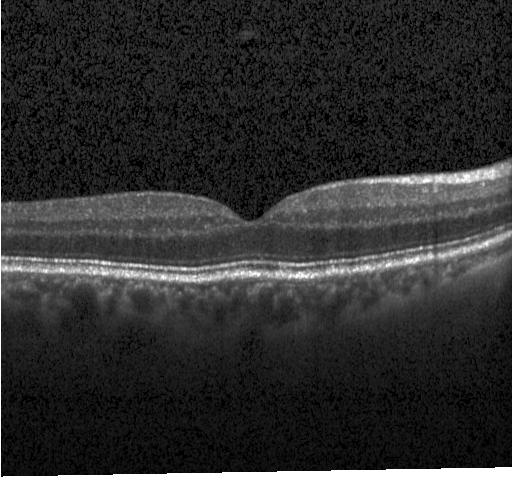
OCT B-scan. Heidelberg Spectralis OCT system. Spectral-domain optical coherence tomography. Horizontal scan through the fovea
Finding: no choroidal neovascularization, diabetic macular edema, or drusen.